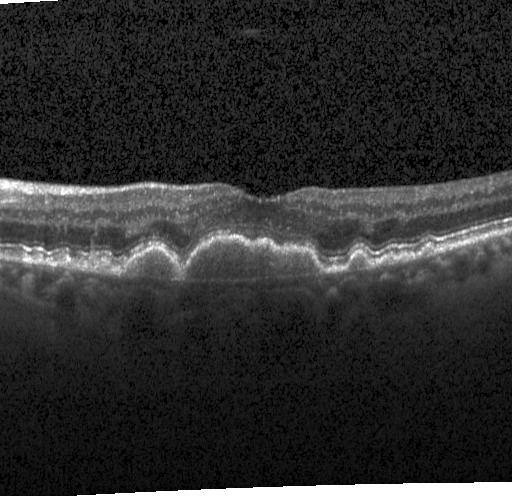 Finding: a choroidal neovascular membrane.